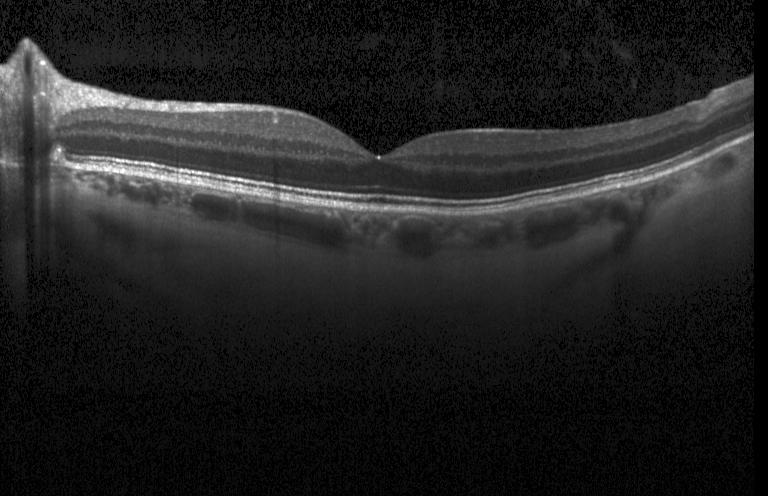 Finding: neither choroidal neovascularization, diabetic macular edema, nor drusen.